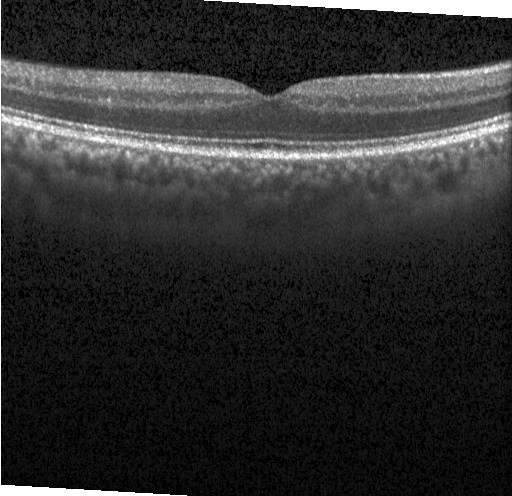 OCT B-scan showing neither choroidal neovascularization, diabetic macular edema, nor drusen.